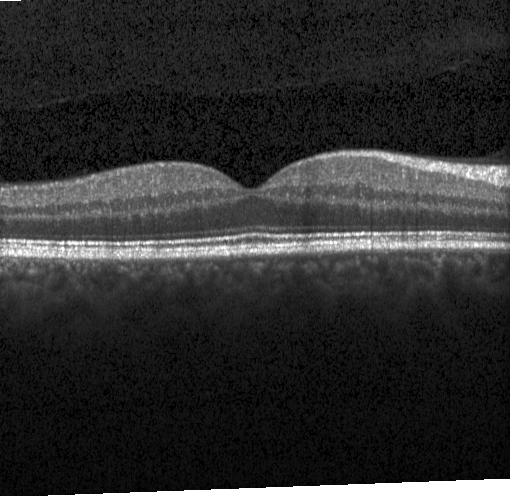 Horizontal scan through the fovea; retinal OCT cross-section; instrument: Heidelberg Spectralis
Neither choroidal neovascularization, diabetic macular edema, nor drusen.